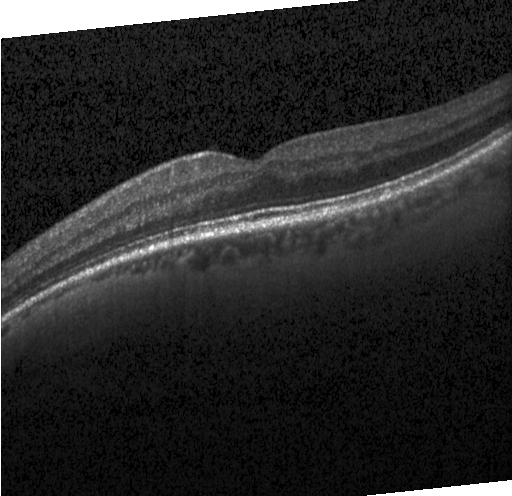 Horizontal scan through the fovea. Spectral-domain optical coherence tomography. Retinal OCT B-scan
Dx: neither choroidal neovascularization, diabetic macular edema, nor drusen.